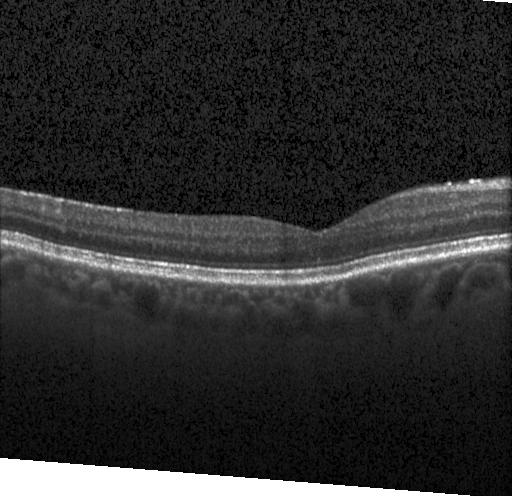

Centered on the fovea · Heidelberg Spectralis · retinal OCT B-scan · spectral-domain optical coherence tomography
Impression: no choroidal neovascularization, diabetic macular edema, or drusen.